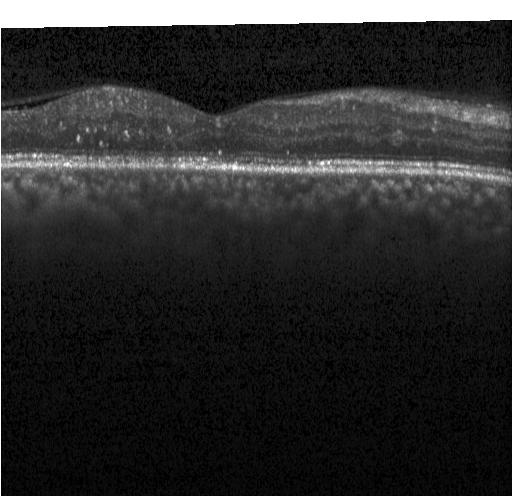 Retinal OCT B-scan — Finding: diabetic macular edema.